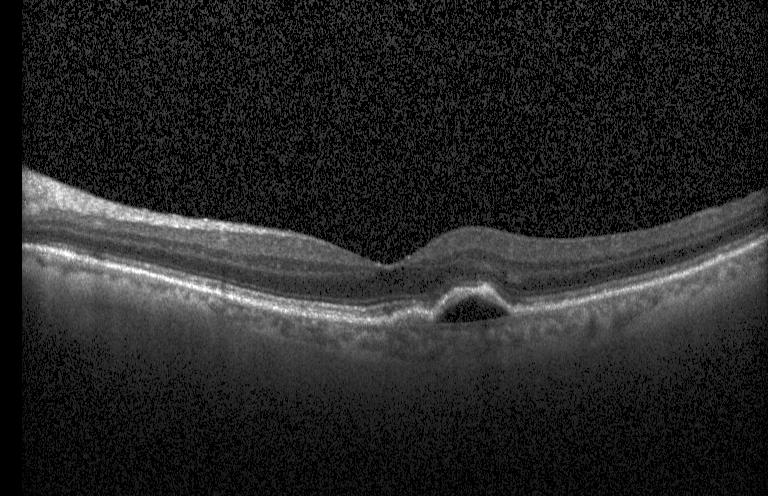 Optical coherence tomography scan. Through the macula — Impression: a choroidal neovascular membrane.